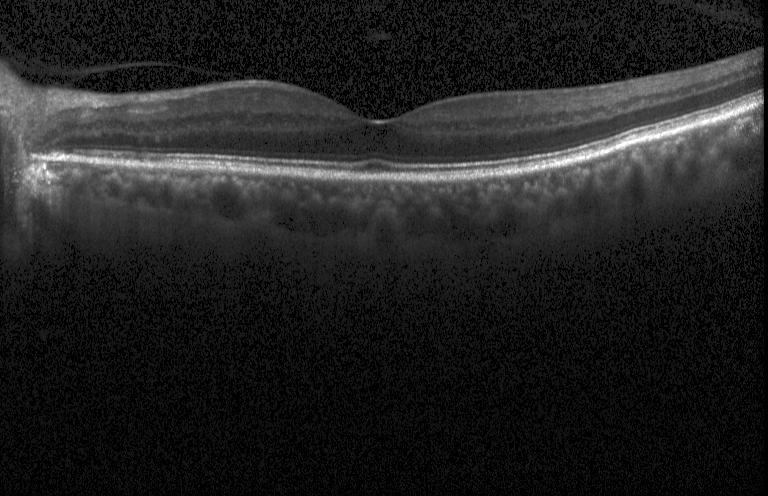 Retinal OCT B-scan · macular scan.
Finding: neither choroidal neovascularization, diabetic macular edema, nor drusen.